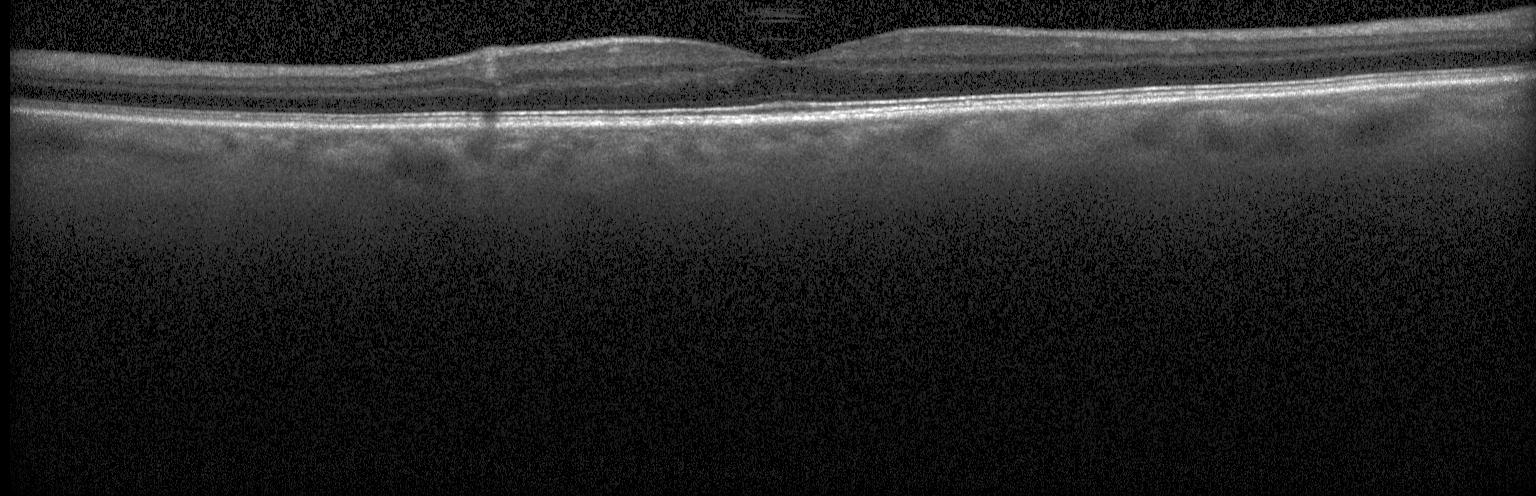
Spectral-domain OCT B-scan: no CNV, no DME, and no drusen.